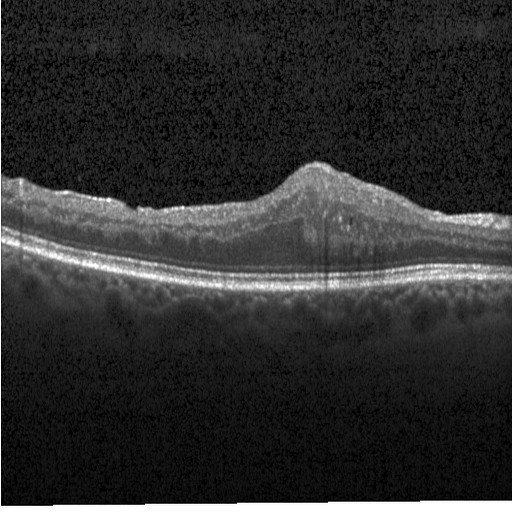
Heidelberg Spectralis OCT system, retinal OCT B-scan, spectral-domain OCT
Finding: DME.